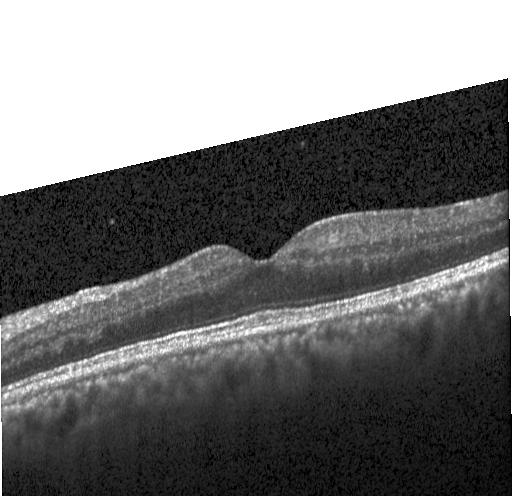

Heidelberg Spectralis · retinal OCT cross-section · macular scan — Neither choroidal neovascularization, diabetic macular edema, nor drusen.